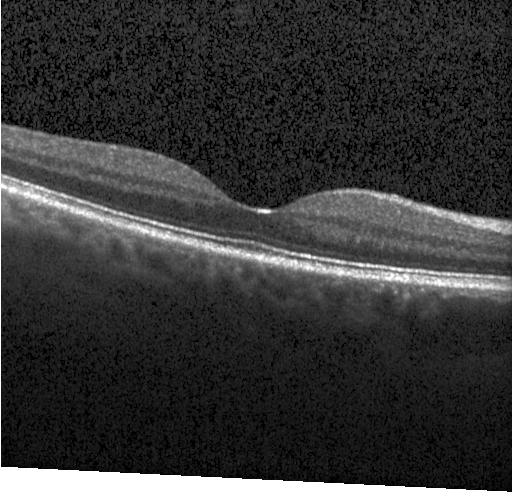 Retinal OCT cross-section · SD-OCT · acquired on a Heidelberg Spectralis · centered on the fovea. The scan shows no choroidal neovascularization, diabetic macular edema, or drusen.